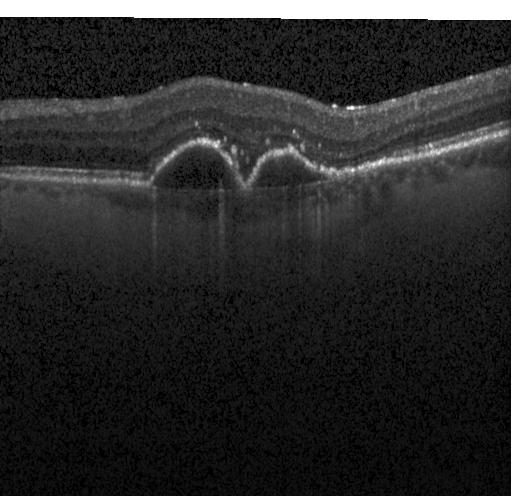

Assessment: choroidal neovascularization (CNV).